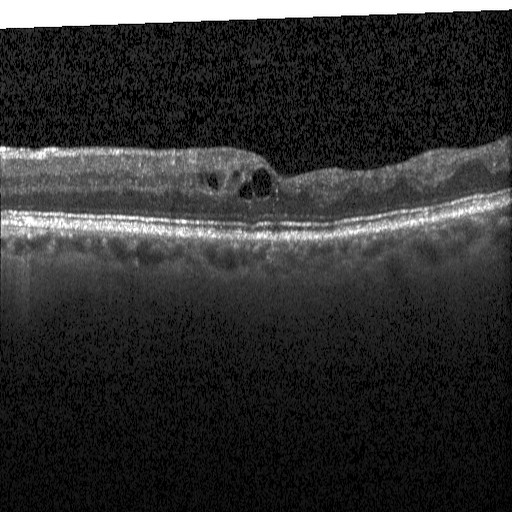
OCT finding: diabetic macular edema (DME).